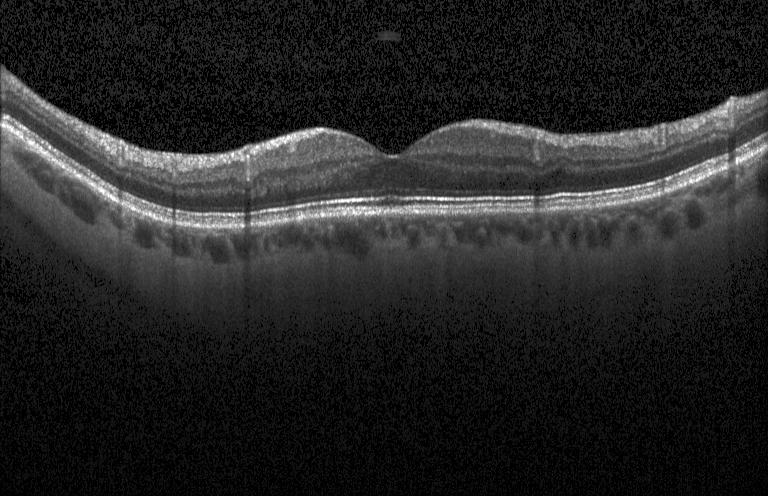 Optical coherence tomography scan
No CNV, DME, or drusen.